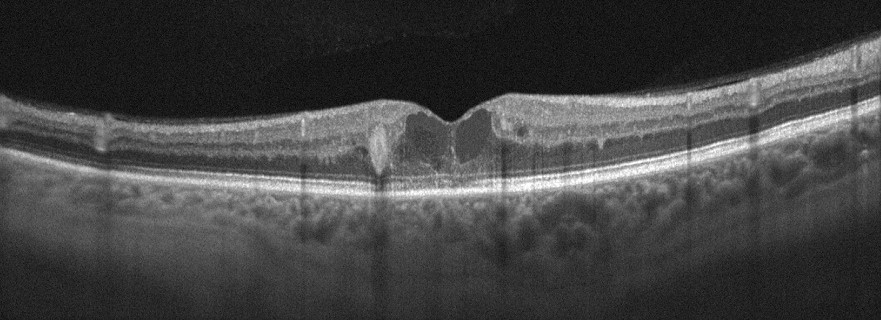
Finding: DME.